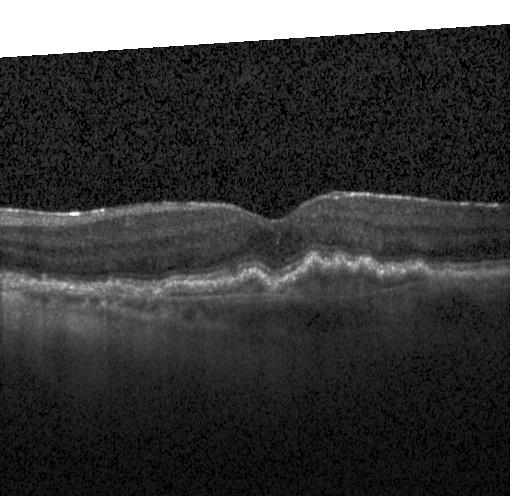 OCT B-scan showing CNV.